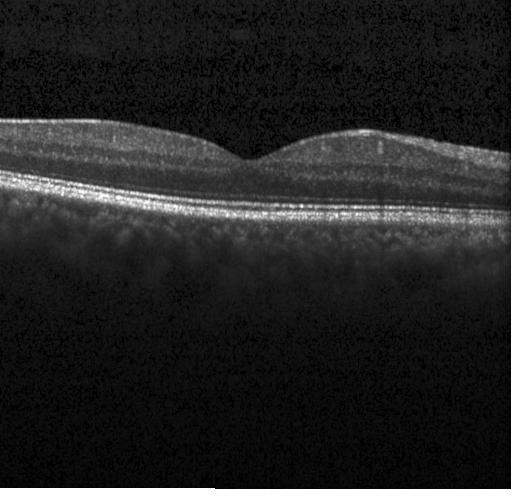
Heidelberg Spectralis OCT system. OCT B-scan.
Macular OCT: no choroidal neovascularization, no diabetic macular edema, and no drusen.